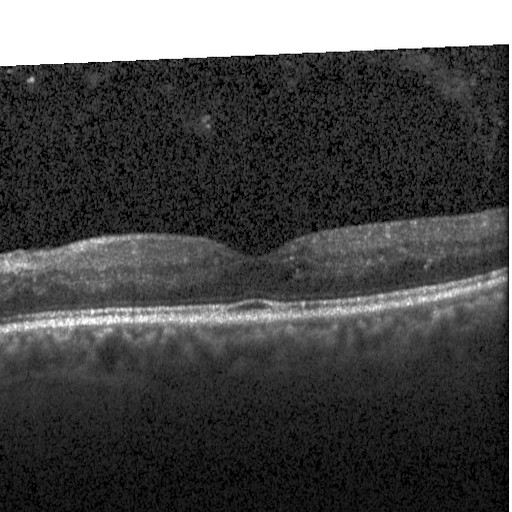

Heidelberg Spectralis OCT system. Retinal OCT cross-section. SD-OCT. Fovea-centered.
Finding: DME.